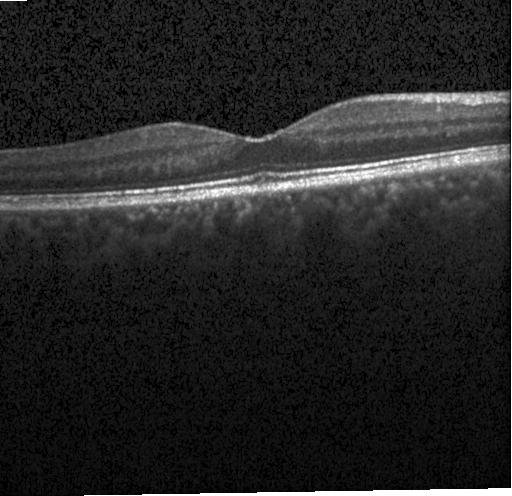

Retinal OCT cross-section, through the macula. Finding: no CNV, DME, or drusen.